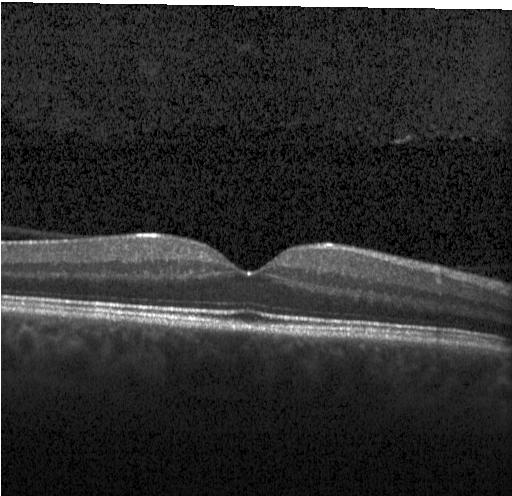 Centered on the fovea; SD-OCT; retinal OCT B-scan; acquired on a Heidelberg Spectralis. Diagnosis: no evidence of choroidal neovascularization, diabetic macular edema, or drusen.